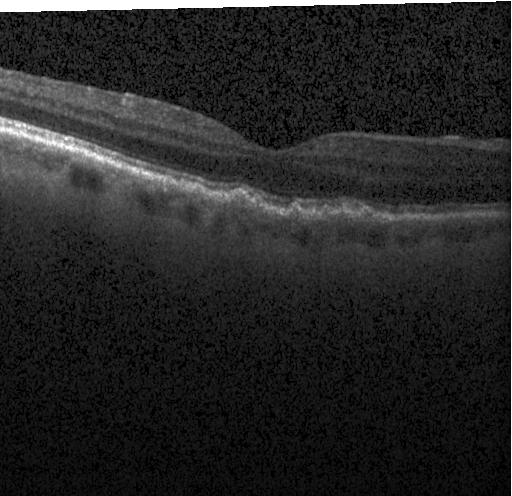
OCT B-scan. This B-scan demonstrates sub-RPE drusenoid deposits.